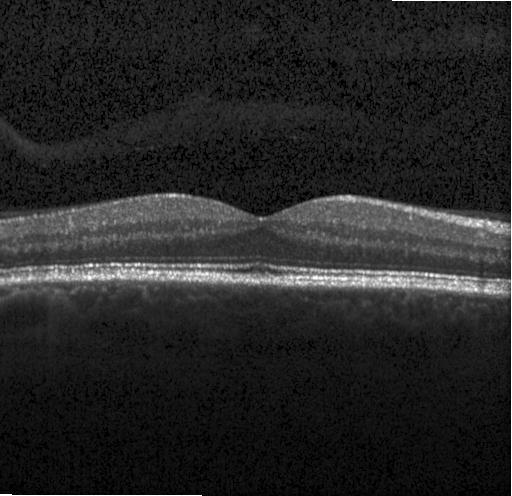 Optical coherence tomography scan — Diagnosis: neither choroidal neovascularization, diabetic macular edema, nor drusen.